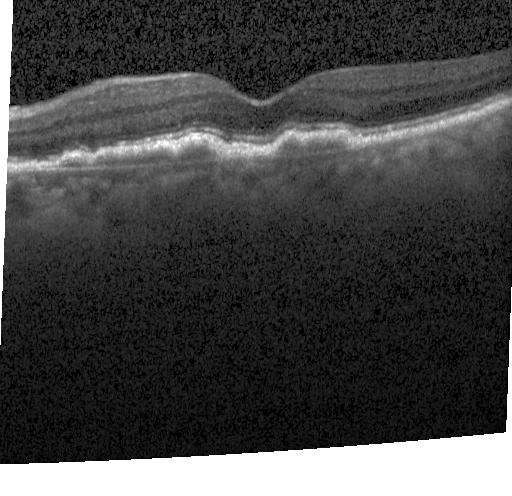
Diagnosis: a choroidal neovascular membrane.